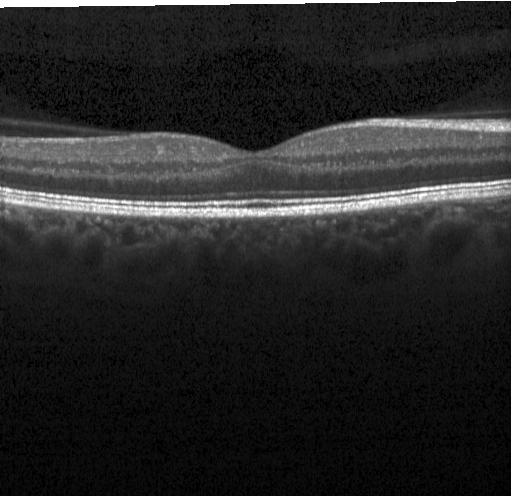
Optical coherence tomography B-scan
Assessment: no choroidal neovascularization, diabetic macular edema, or drusen.